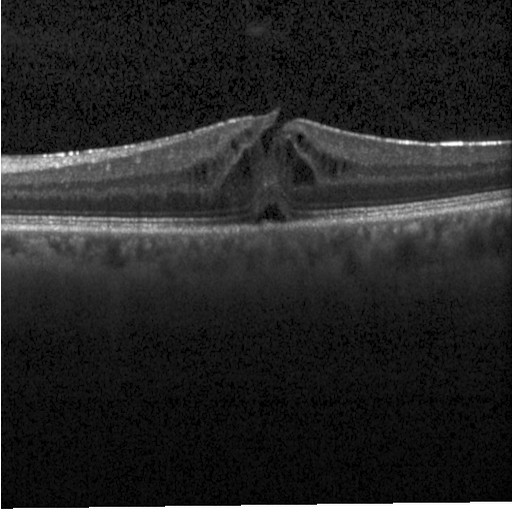
Heidelberg Spectralis OCT system · spectral-domain optical coherence tomography · retinal OCT cross-section · fovea-centered.
Diagnosis: diabetic macular edema (DME).